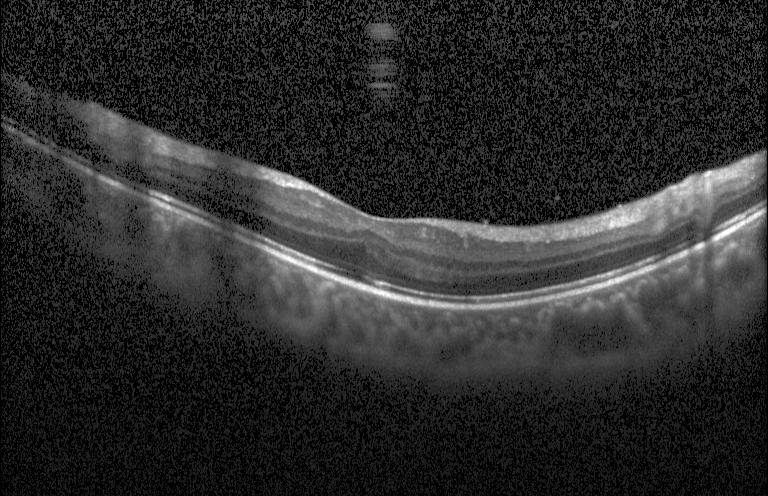

Instrument: Heidelberg Spectralis, OCT line scan, macular scan
Impression: no choroidal neovascularization, no diabetic macular edema, and no drusen.